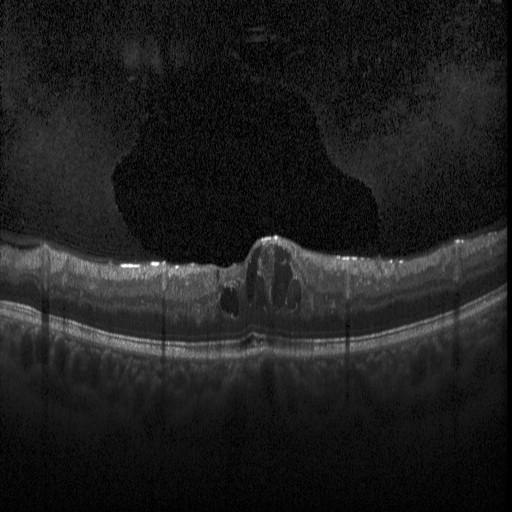

Assessment: DME.